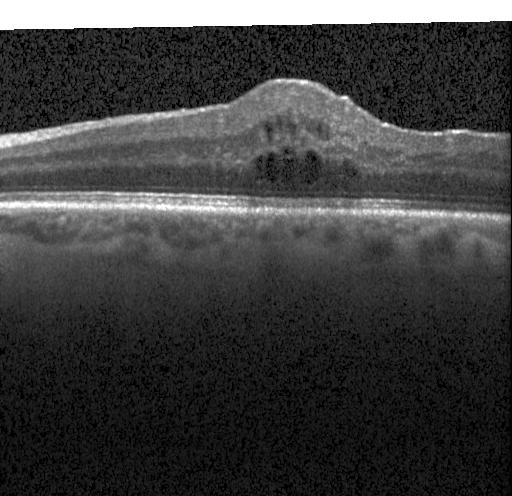
This B-scan demonstrates DME.